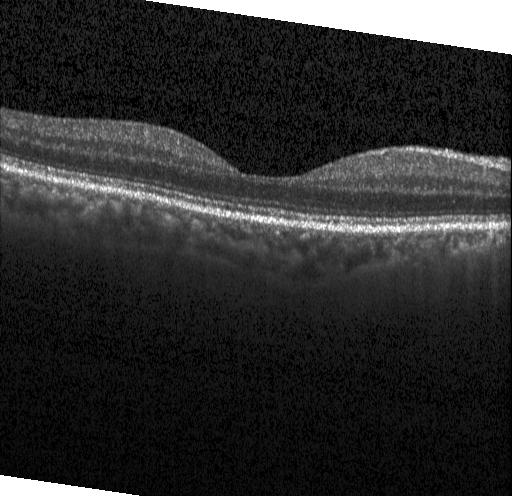 Instrument: Heidelberg Spectralis, through the macula, optical coherence tomography scan. Impression: no choroidal neovascularization, diabetic macular edema, or drusen.